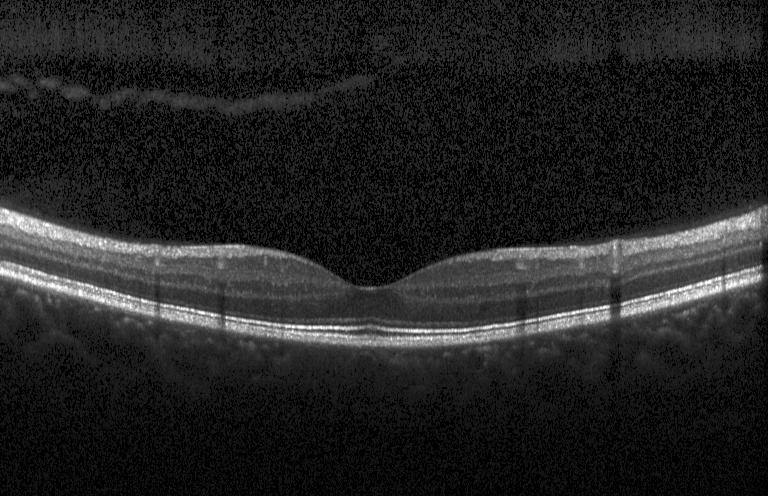
OCT B-scan, centered on the fovea. The scan shows no evidence of CNV, DME, or drusen.